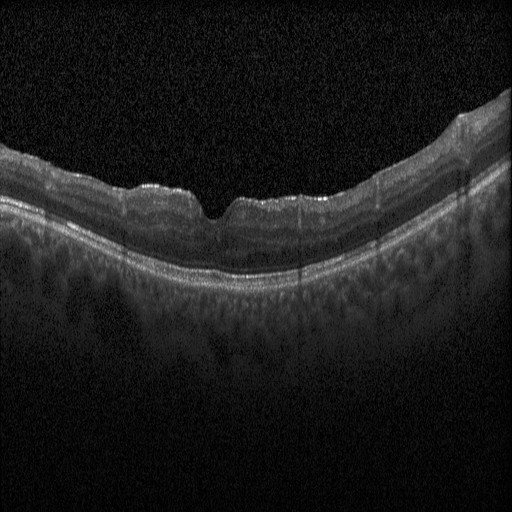
Optical coherence tomography scan.
Finding: diabetic macular edema (DME).